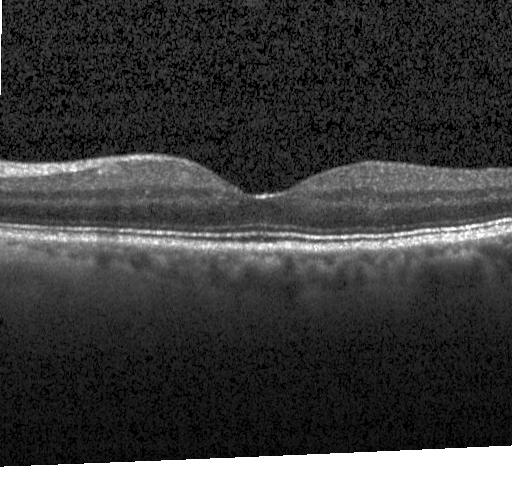
Centered on the fovea, optical coherence tomography scan, instrument: Heidelberg Spectralis.
Finding: no choroidal neovascularization, diabetic macular edema, or drusen.